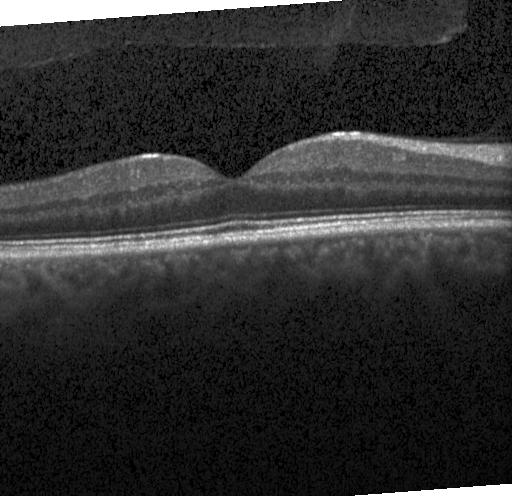 Spectral-domain OCT; OCT line scan; Heidelberg Spectralis OCT system — Impression: no CNV, DME, or drusen.